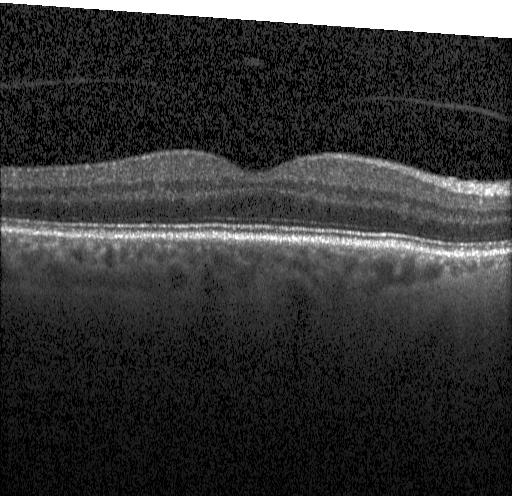 Optical coherence tomography B-scan.
Finding: no evidence of choroidal neovascularization, diabetic macular edema, or drusen.